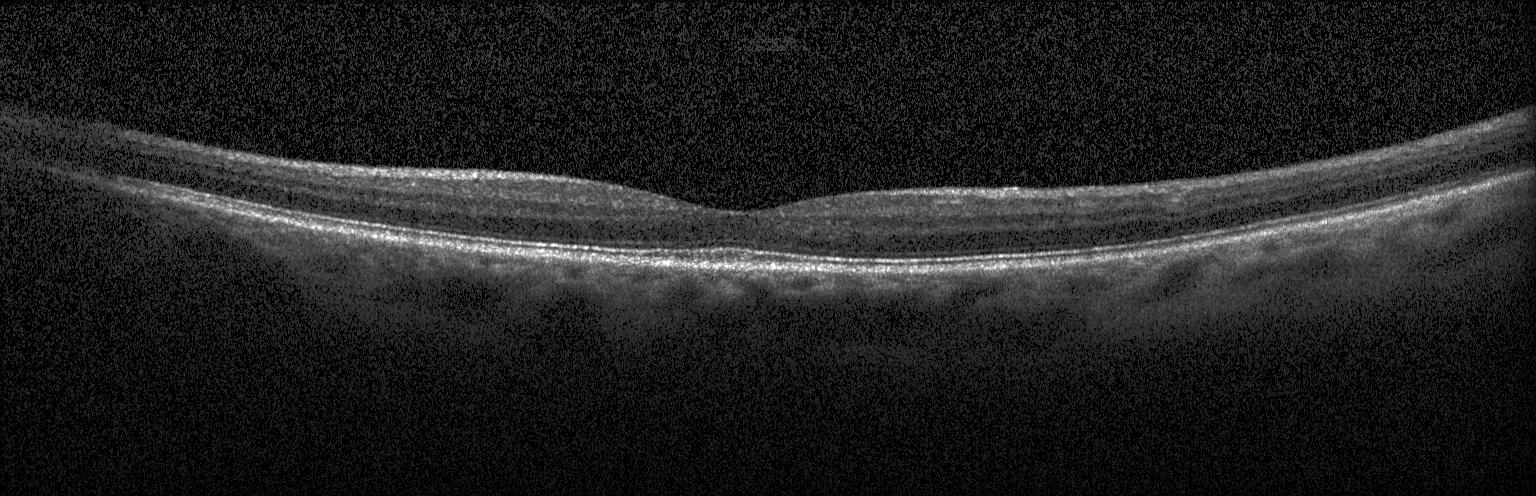

Diagnosis: no choroidal neovascularization, diabetic macular edema, or drusen.